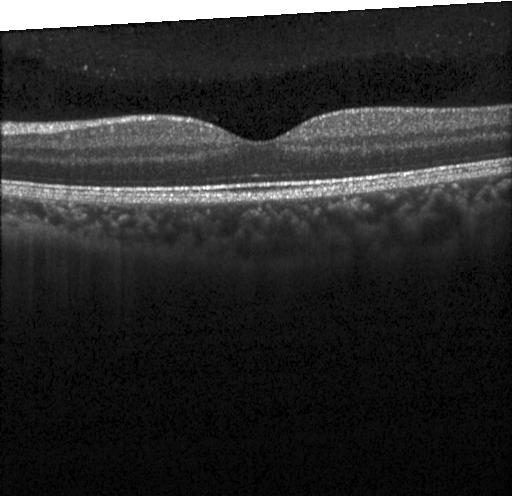 Optical coherence tomography scan
Assessment: no evidence of choroidal neovascularization, diabetic macular edema, or drusen.